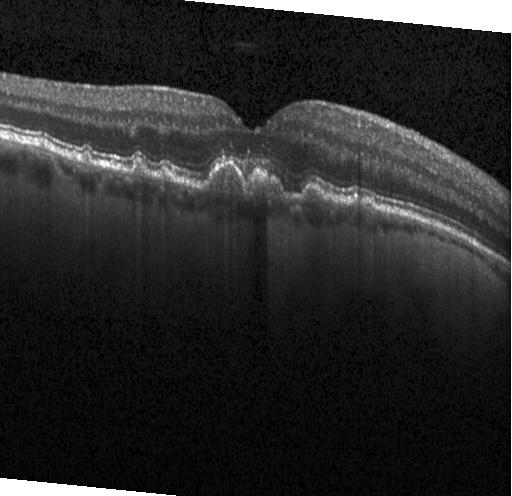 Retinal OCT cross-section showing drusen.